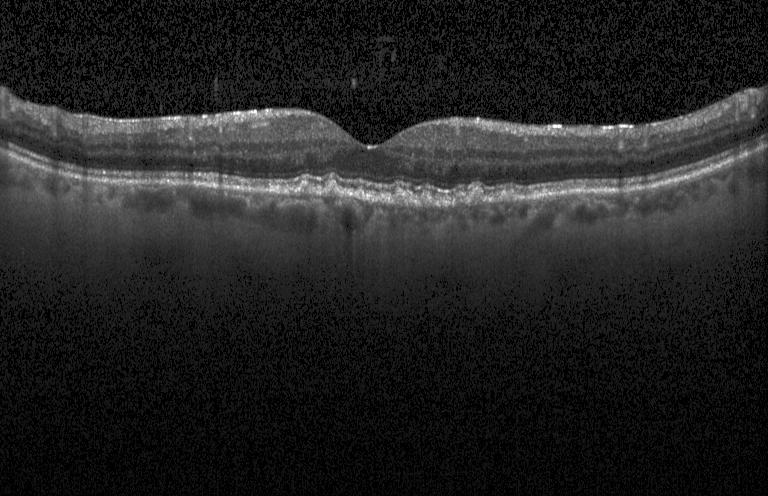
OCT line scan
This B-scan demonstrates drusen.